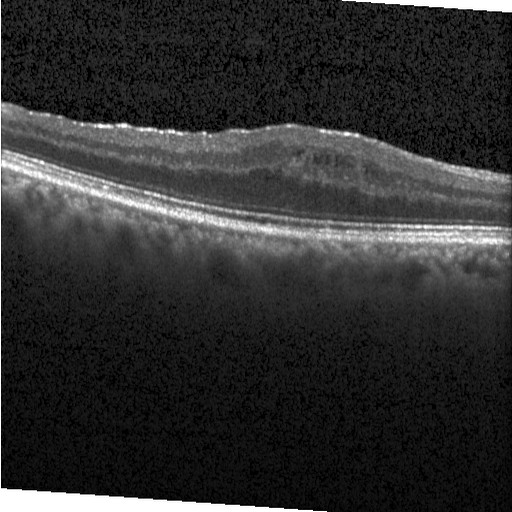

OCT finding: diabetic macular edema.